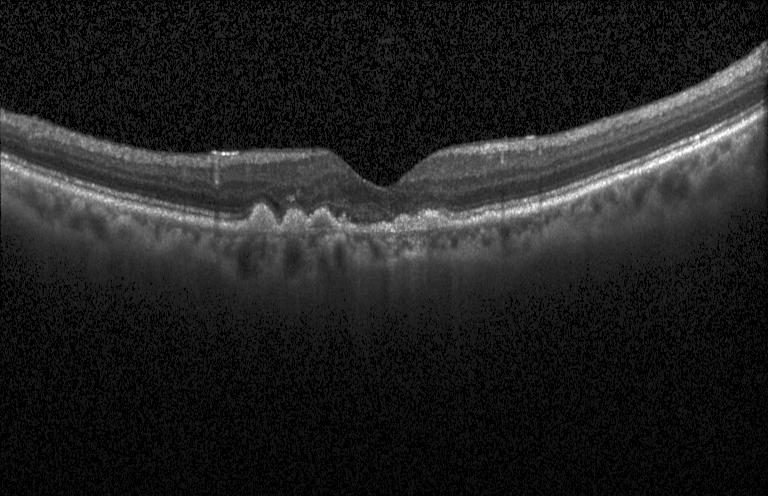
OCT line scan · Heidelberg Spectralis
Assessment: a choroidal neovascular membrane.